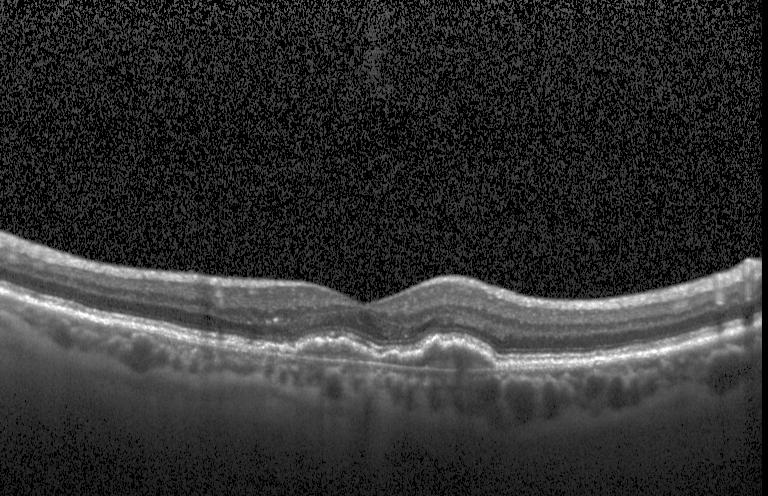 Retinal OCT B-scan; macular scan; acquired on a Heidelberg Spectralis — Finding: choroidal neovascularization (CNV).